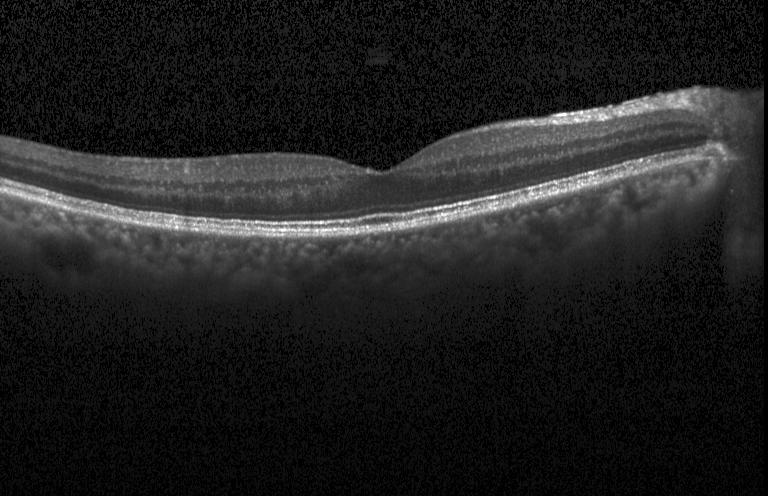
Impression: no choroidal neovascularization, no diabetic macular edema, and no drusen.